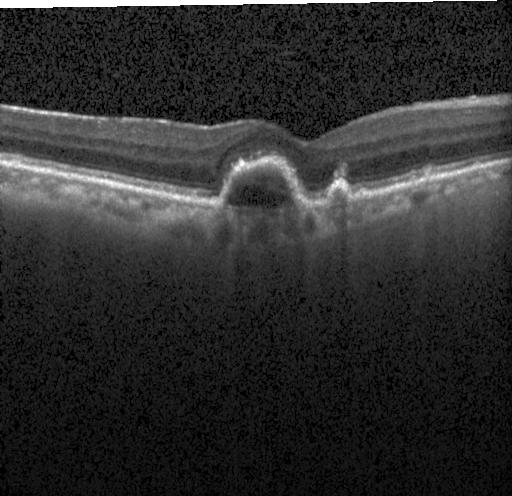 Fovea-centered, spectral-domain OCT, retinal OCT cross-section — Dx: a choroidal neovascular membrane.